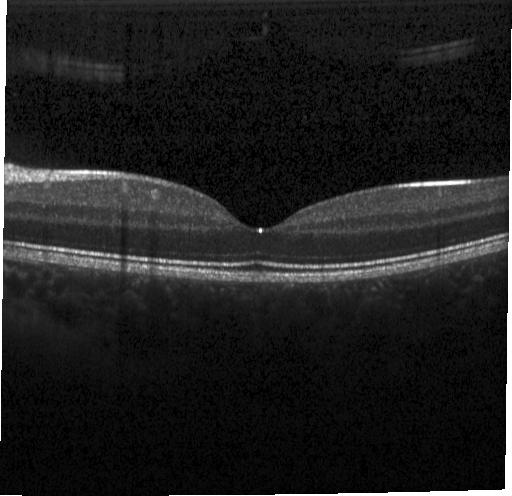

Diagnosis: no choroidal neovascularization, diabetic macular edema, or drusen.